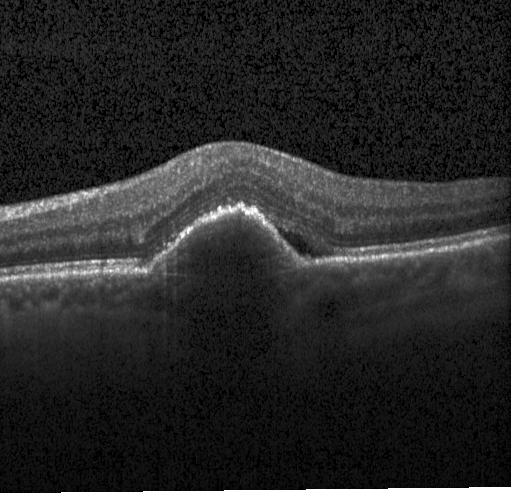

A choroidal neovascular membrane.